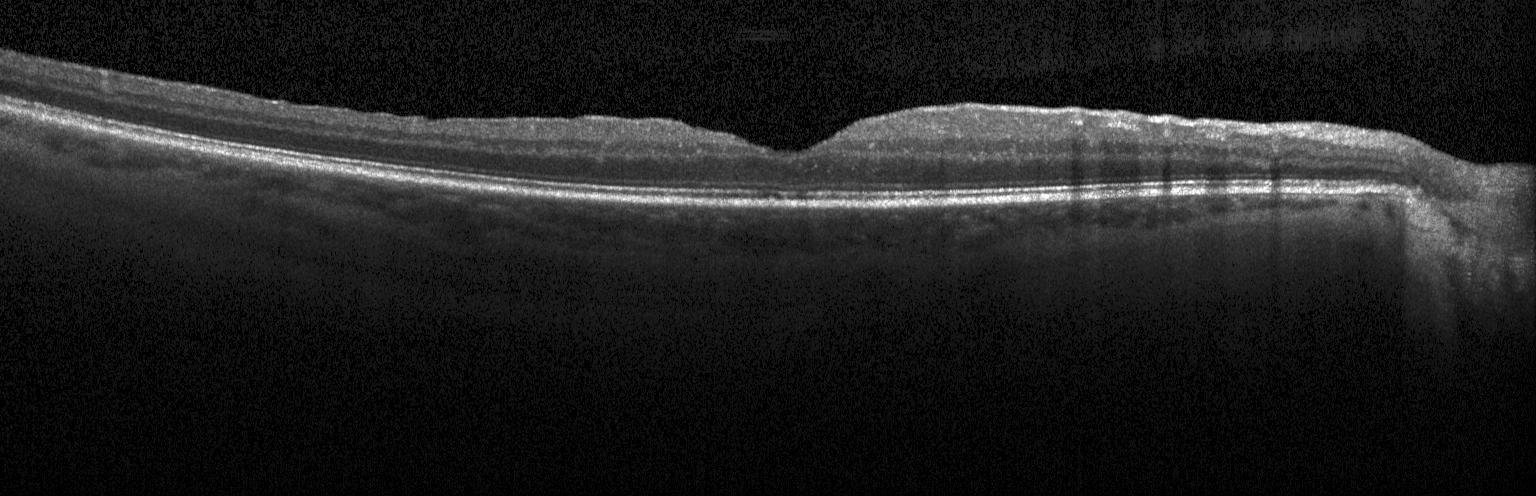 Acquired on a Heidelberg Spectralis, spectral-domain optical coherence tomography, through the macula, optical coherence tomography B-scan
Dx: no evidence of CNV, DME, or drusen.